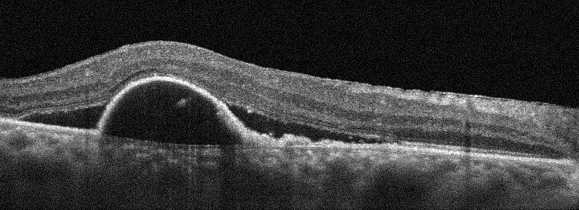
Right eye; retinal OCT cross-section.
Finding: AMD.